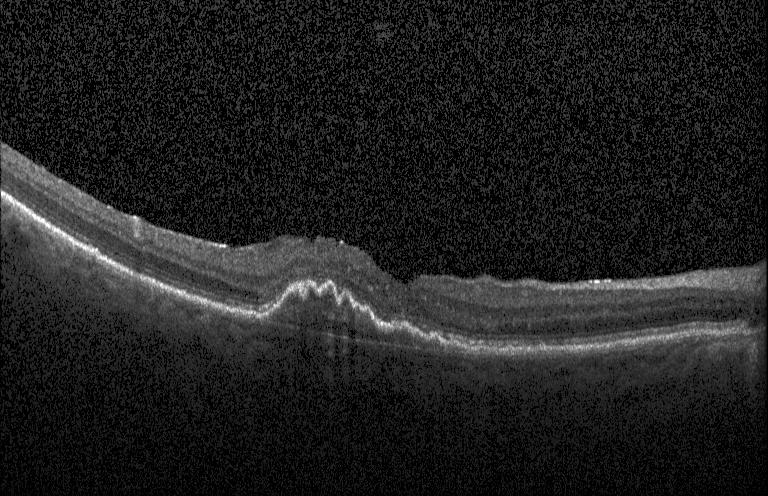 Retinal OCT B-scan; instrument: Heidelberg Spectralis; macular scan; spectral-domain optical coherence tomography. Macular OCT: a choroidal neovascular membrane.